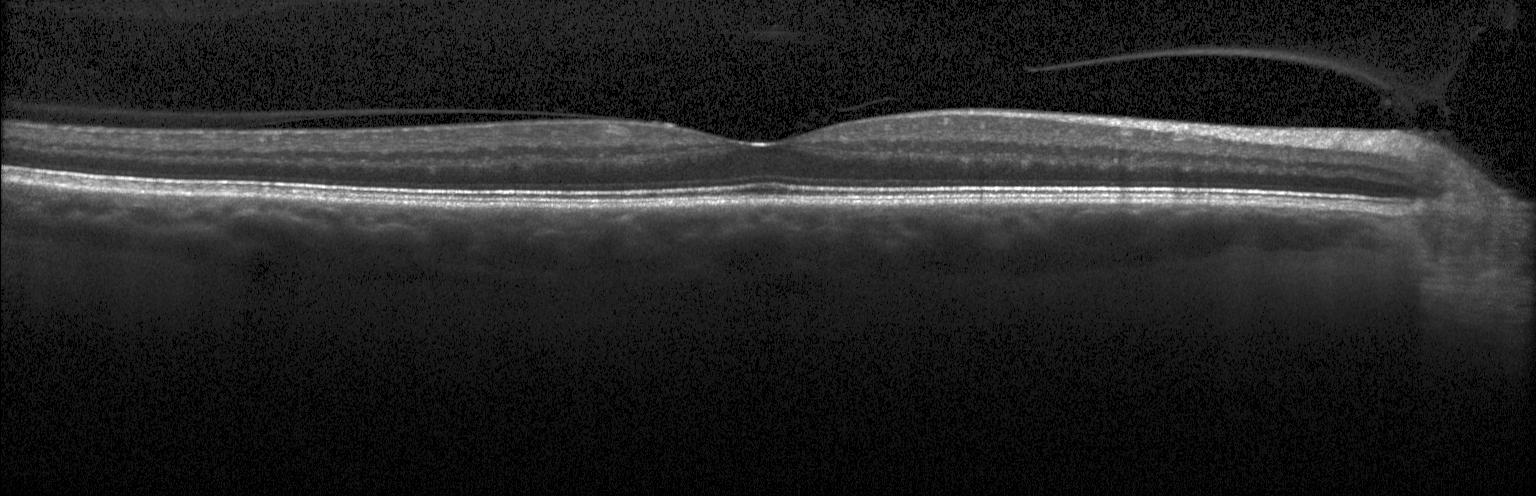

Optical coherence tomography scan — Impression: no CNV, no DME, and no drusen.